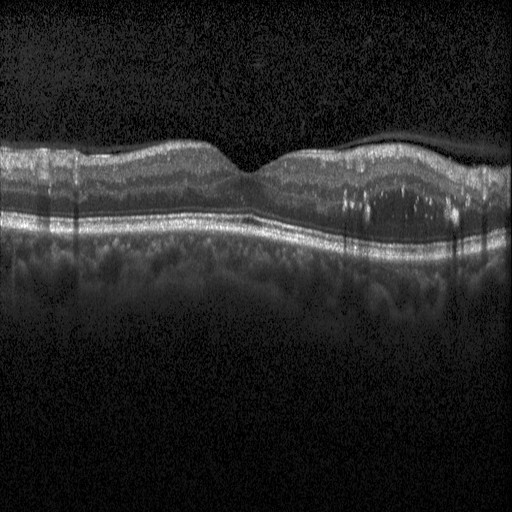

Instrument: Heidelberg Spectralis · OCT B-scan — Diagnosis: diabetic macular edema.